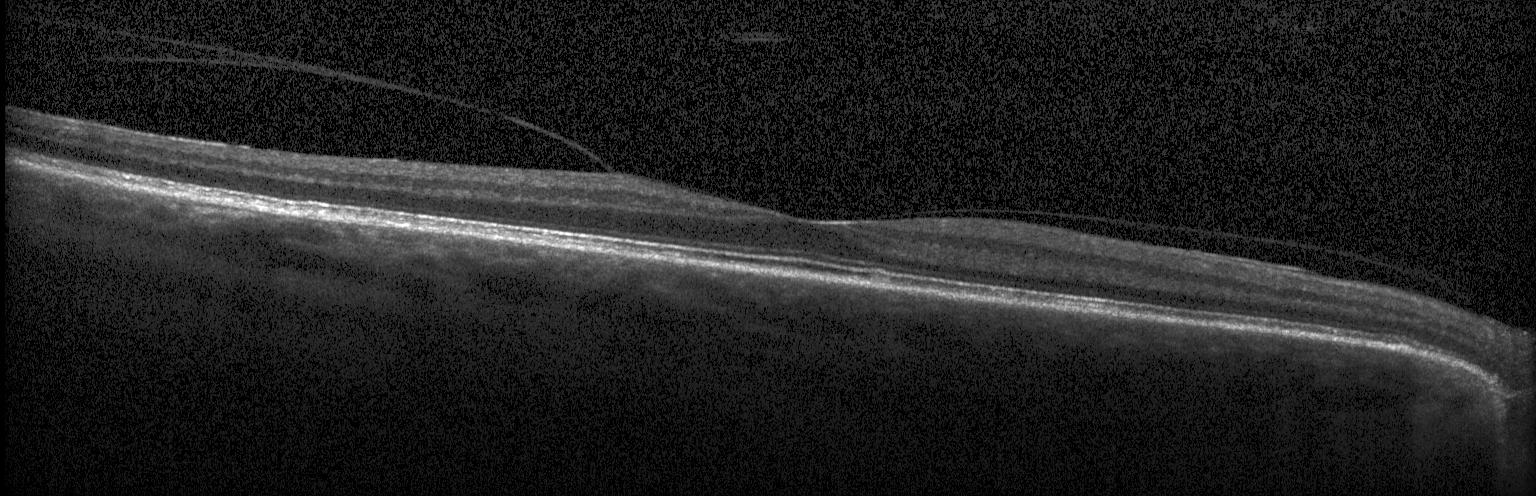

OCT line scan; through the macula — The scan shows no evidence of choroidal neovascularization, diabetic macular edema, or drusen.